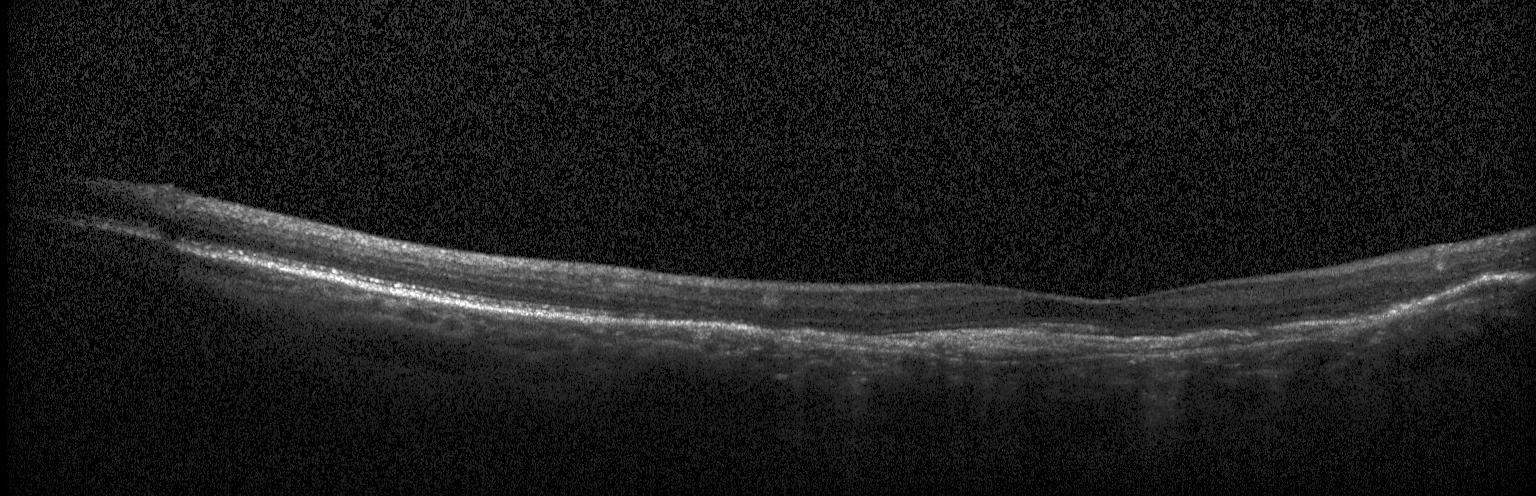
Optical coherence tomography B-scan.
This B-scan demonstrates choroidal neovascularization (CNV).